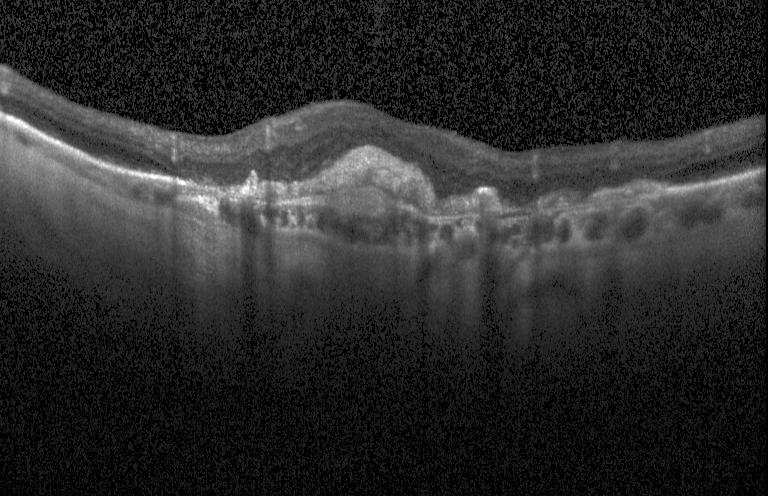 Heidelberg Spectralis. Retinal OCT cross-section. Impression: a choroidal neovascular membrane.